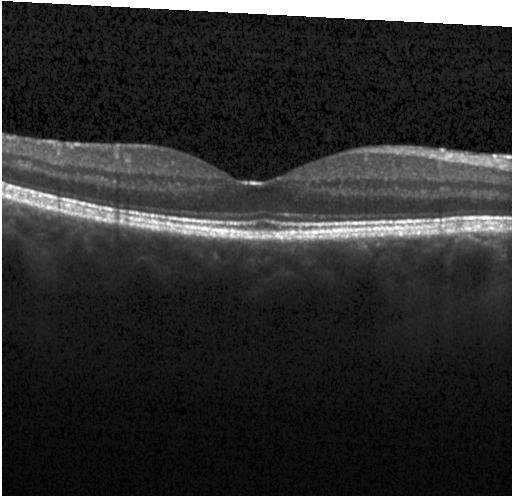 Macular OCT demonstrating neither CNV, DME, nor drusen.